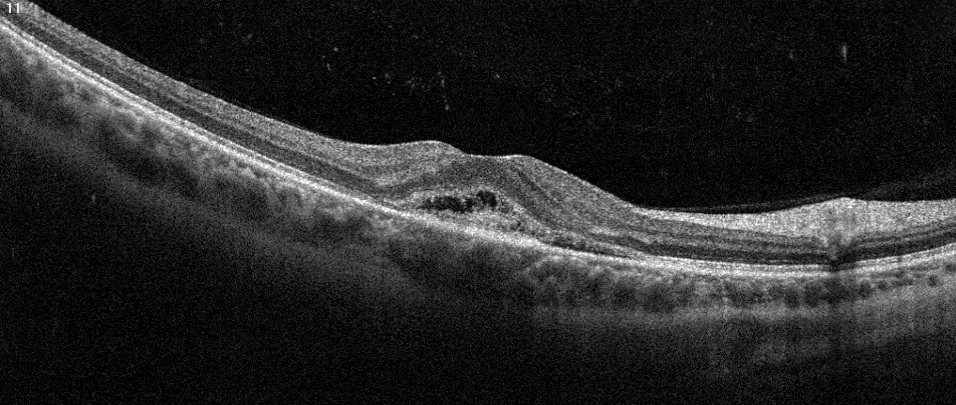 Diagnosis: AMD.